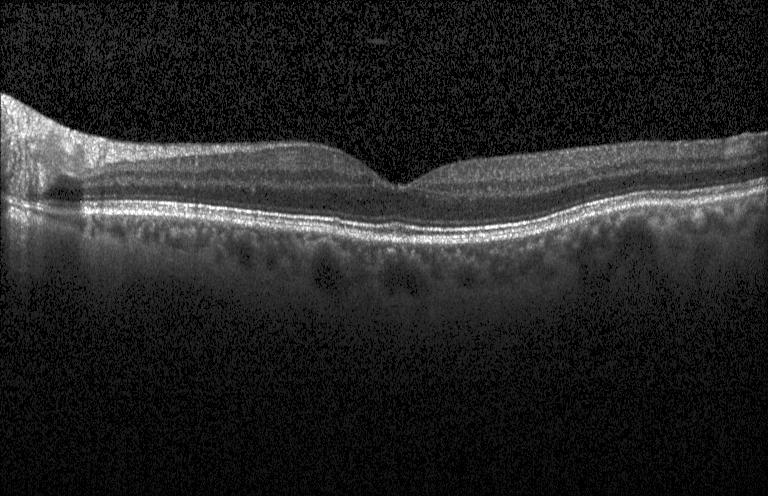 Spectral-domain OCT · centered on the fovea · instrument: Heidelberg Spectralis · retinal OCT cross-section. Impression: neither CNV, DME, nor drusen.